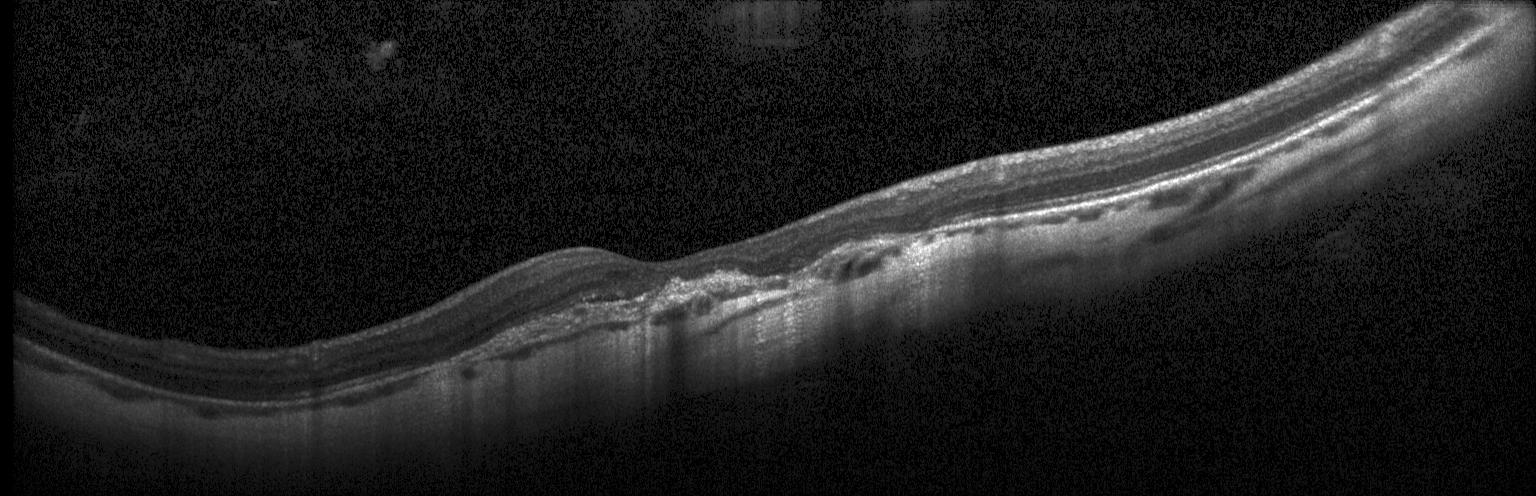 Finding: choroidal neovascularization (CNV).